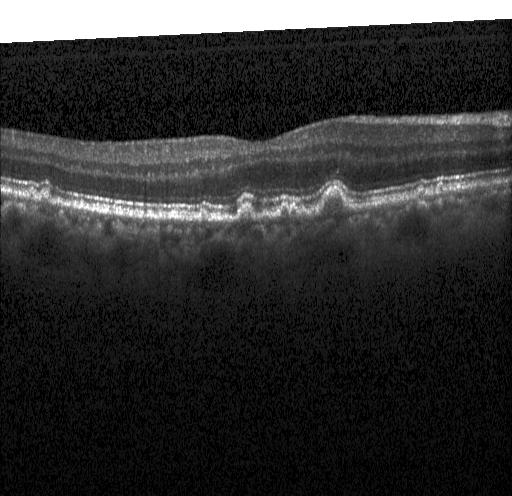

Retinal OCT B-scan · spectral-domain optical coherence tomography · instrument: Heidelberg Spectralis.
OCT finding: multiple drusen.